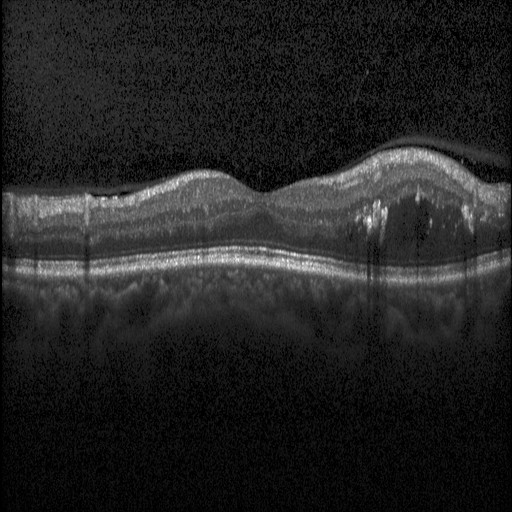 Instrument: Heidelberg Spectralis; spectral-domain OCT; optical coherence tomography B-scan; centered on the fovea. Assessment: diabetic macular edema (DME).